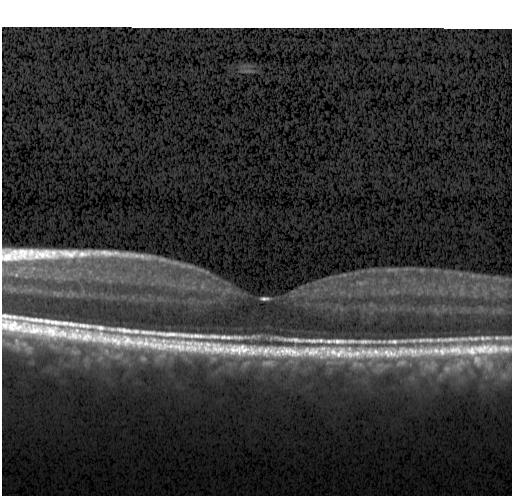

This B-scan demonstrates neither choroidal neovascularization, diabetic macular edema, nor drusen.